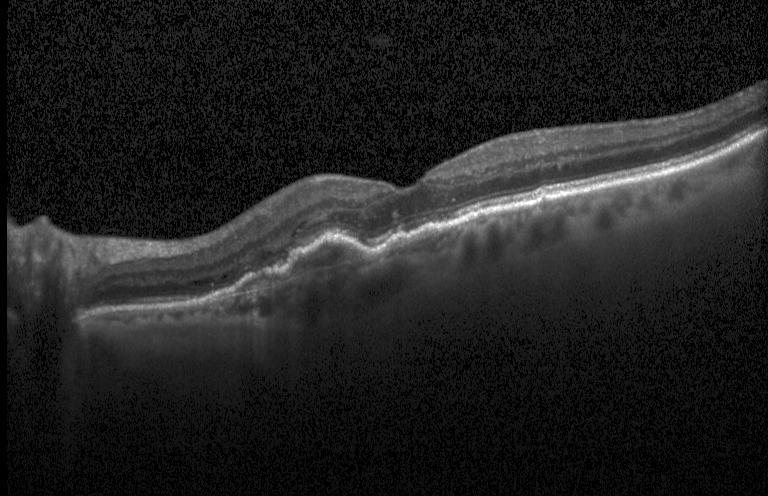

Instrument: Heidelberg Spectralis. Retinal OCT cross-section
Finding: a choroidal neovascular membrane.